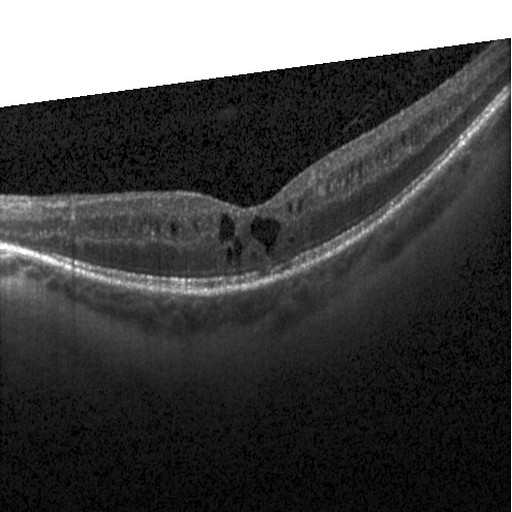

DME.